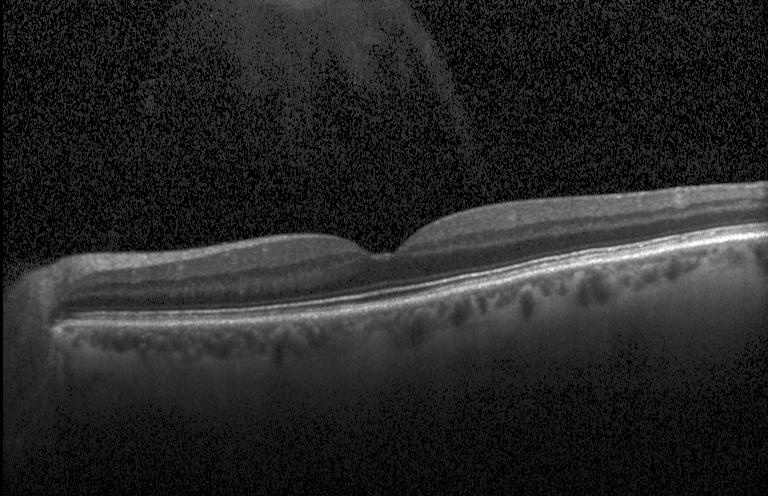
Retinal OCT cross-section showing neither CNV, DME, nor drusen.